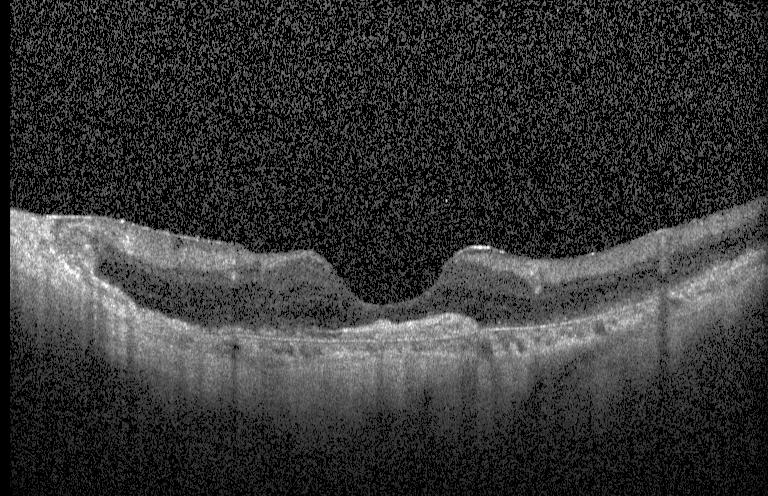 Assessment: CNV.